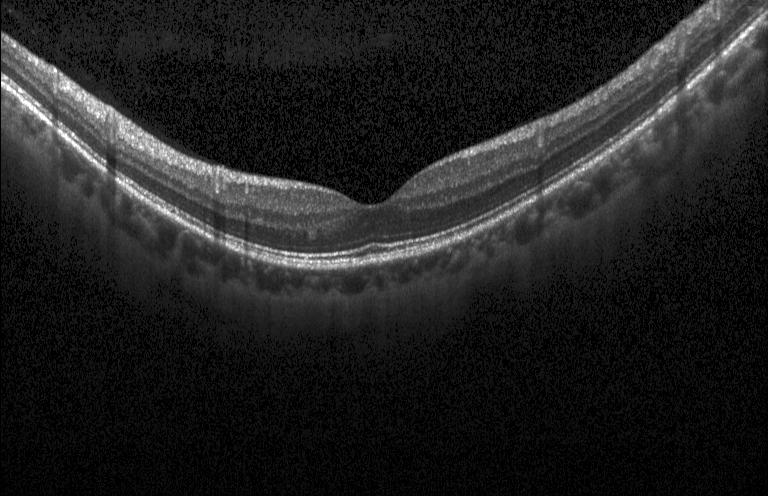

Optical coherence tomography B-scan
Assessment: no choroidal neovascularization, no diabetic macular edema, and no drusen.